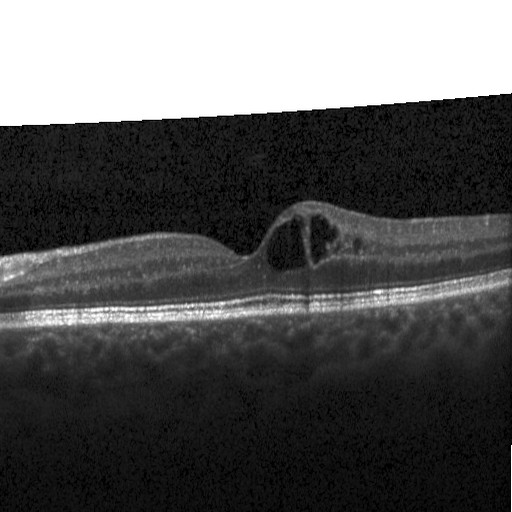

OCT line scan, macular scan
Macular OCT: diabetic macular edema (DME).